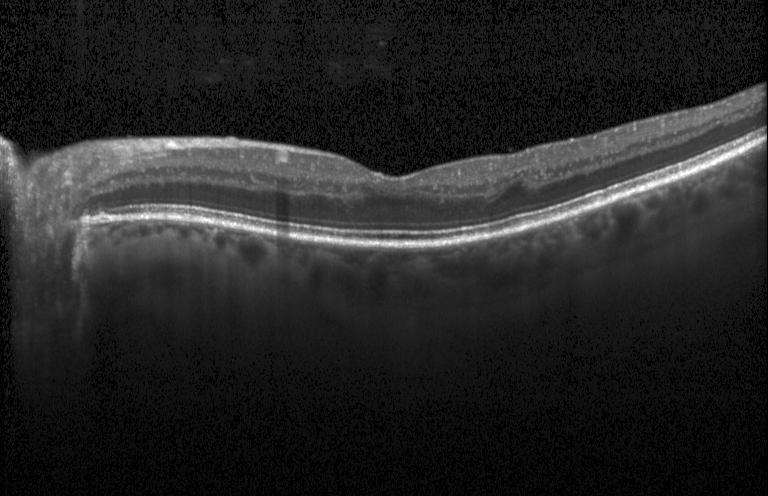 No choroidal neovascularization, diabetic macular edema, or drusen.